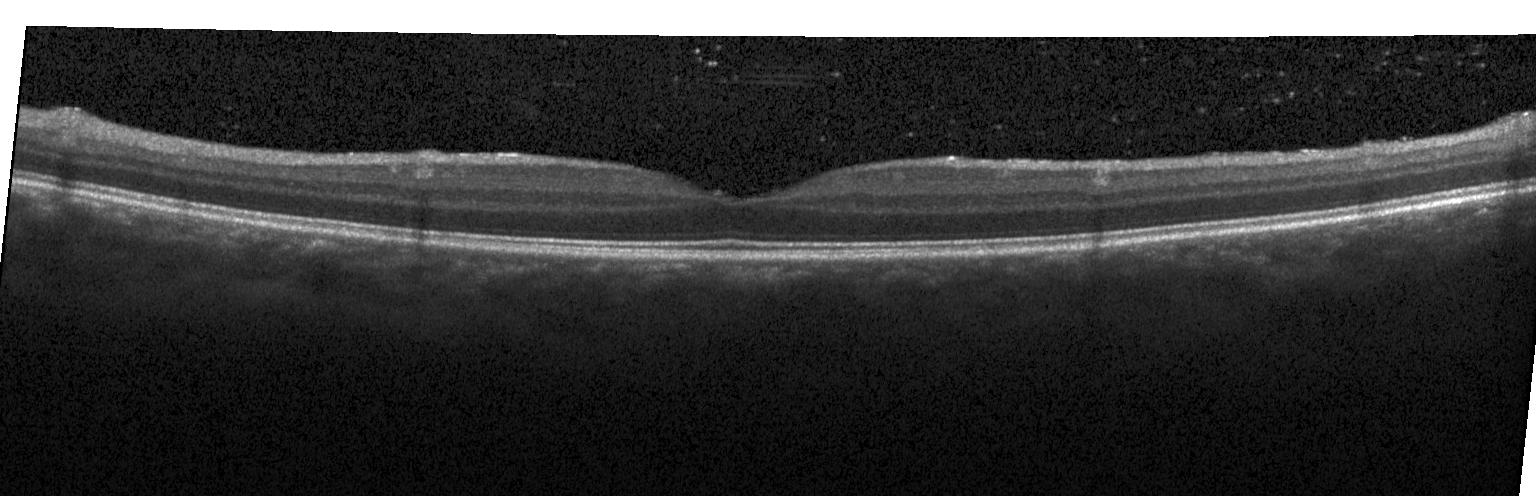 Retinal OCT cross-section. Acquired on a Heidelberg Spectralis. Fovea-centered — Assessment: neither choroidal neovascularization, diabetic macular edema, nor drusen.